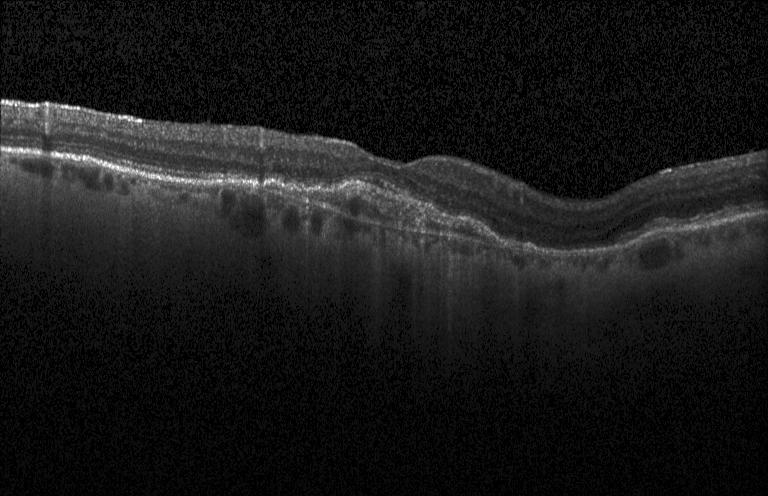

OCT B-scan showing a choroidal neovascular membrane.